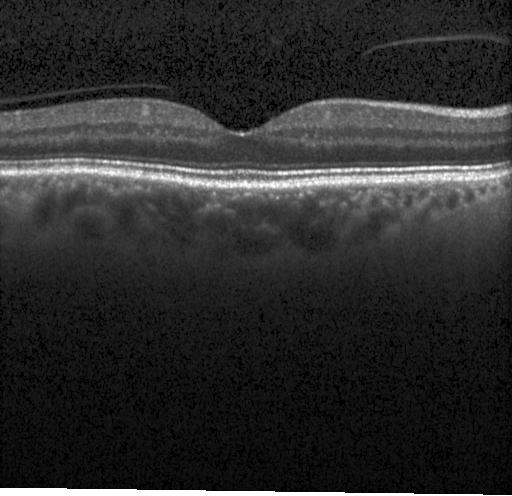

Retinal OCT cross-section.
Finding: neither choroidal neovascularization, diabetic macular edema, nor drusen.